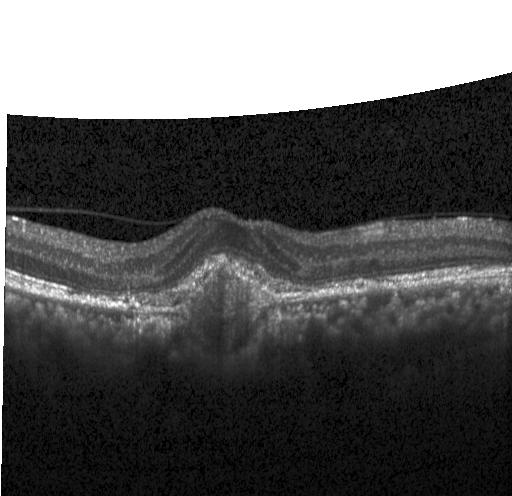 OCT finding: choroidal neovascularization.